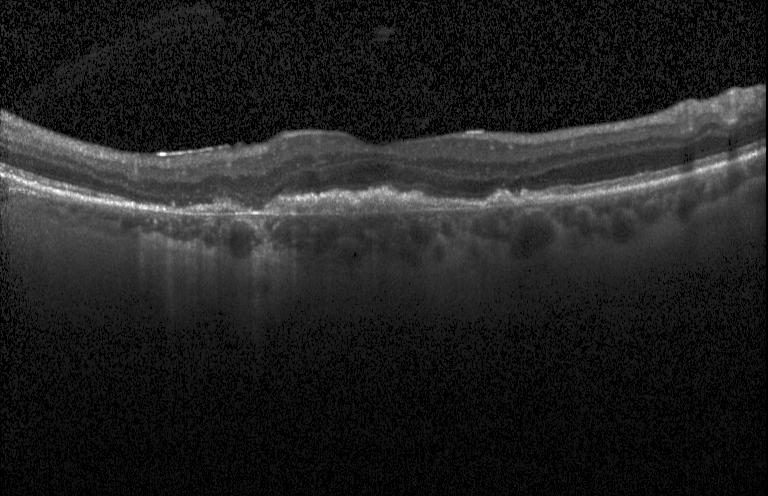
Impression: CNV.